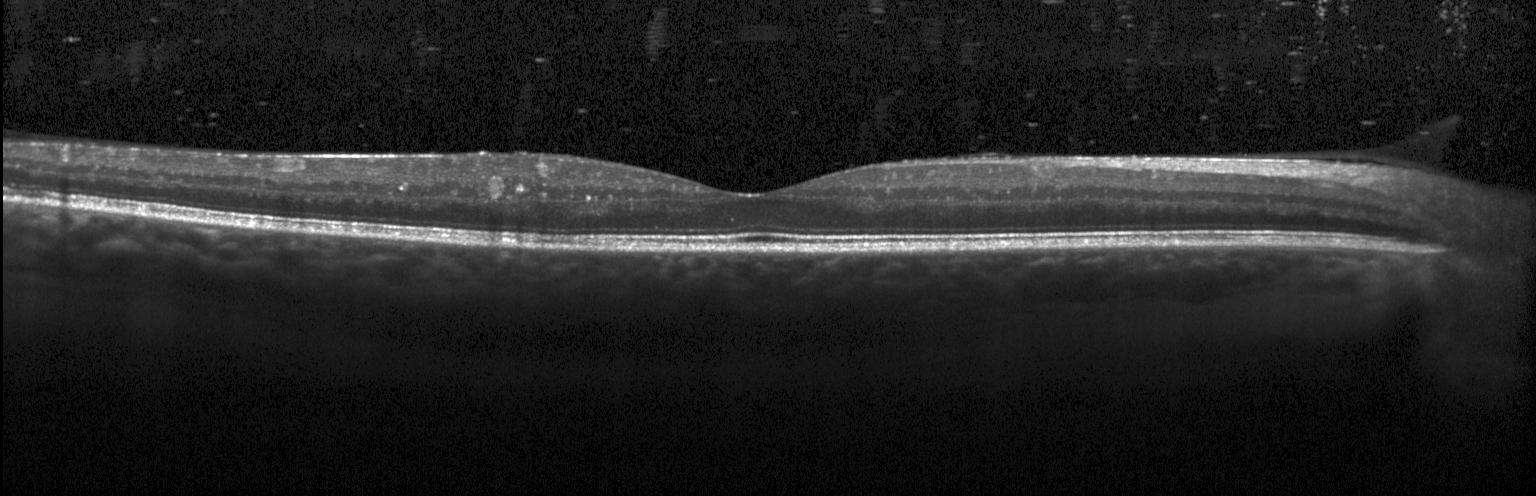

OCT finding: no choroidal neovascularization, no diabetic macular edema, and no drusen.